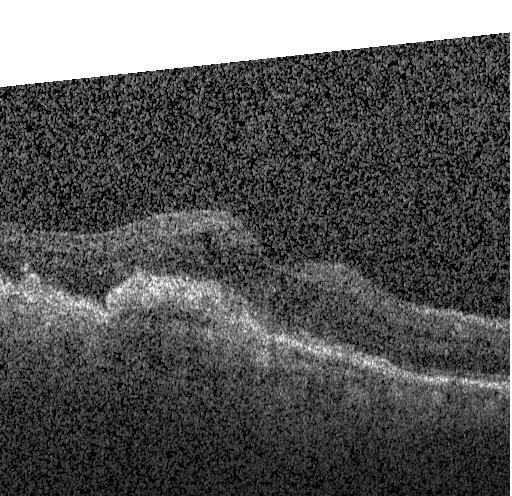 Macular OCT: a choroidal neovascular membrane.